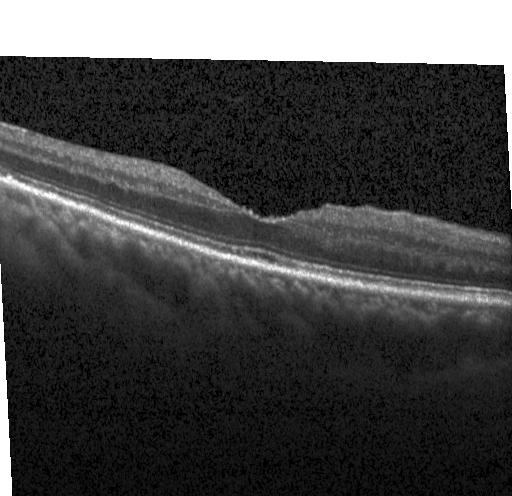

Spectral-domain OCT · centered on the fovea · acquired on a Heidelberg Spectralis · OCT B-scan.
Macular OCT: no choroidal neovascularization, diabetic macular edema, or drusen.